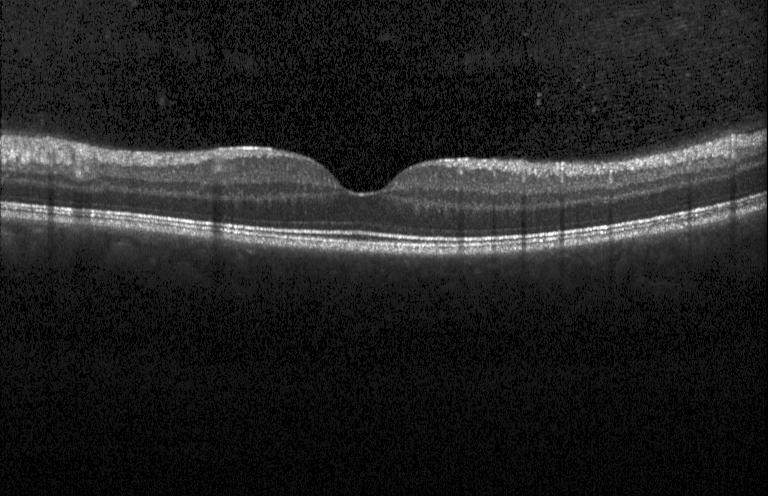
Diagnosis: neither CNV, DME, nor drusen.